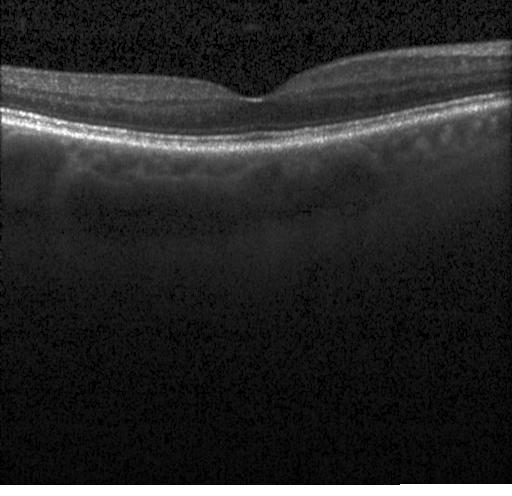

OCT line scan, acquired on a Heidelberg Spectralis, spectral-domain optical coherence tomography. Finding: no evidence of CNV, DME, or drusen.